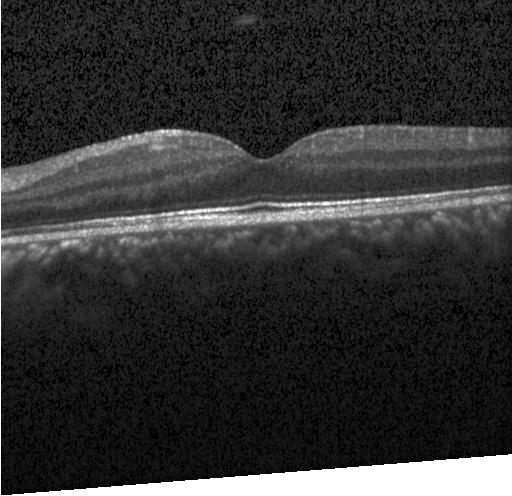
Dx: no choroidal neovascularization, no diabetic macular edema, and no drusen.